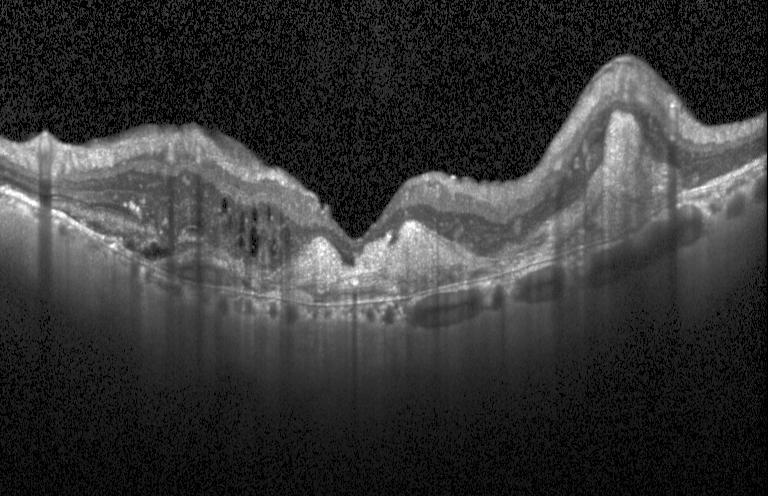
SD-OCT. Through the macula. Optical coherence tomography scan.
This B-scan demonstrates a choroidal neovascular membrane.